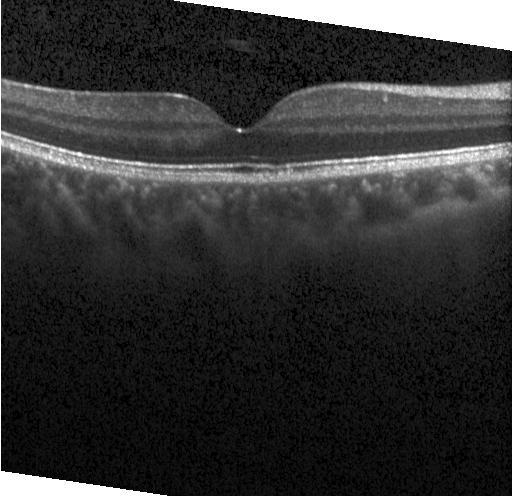 Retinal OCT cross-section showing neither choroidal neovascularization, diabetic macular edema, nor drusen.